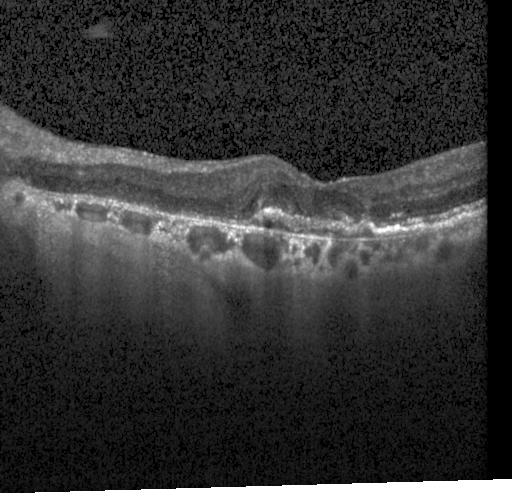
Centered on the fovea. Instrument: Heidelberg Spectralis. Spectral-domain optical coherence tomography. OCT line scan.
This B-scan demonstrates a choroidal neovascular membrane.